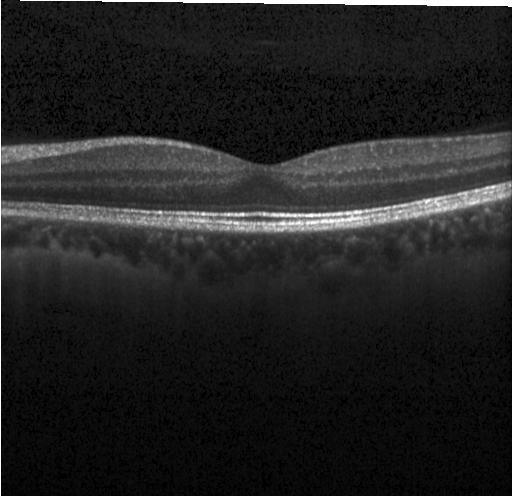
Spectral-domain OCT B-scan: no evidence of choroidal neovascularization, diabetic macular edema, or drusen.